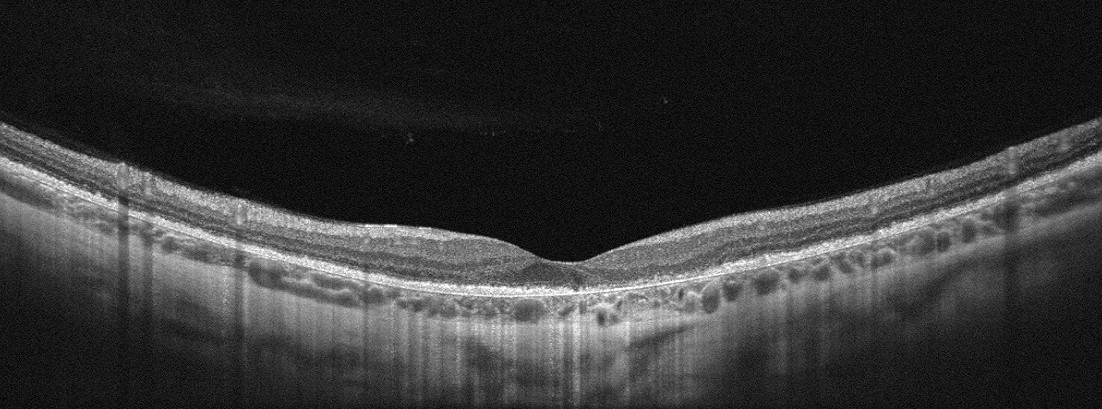

Optical coherence tomography B-scan
Assessment: age-related macular degeneration (AMD).